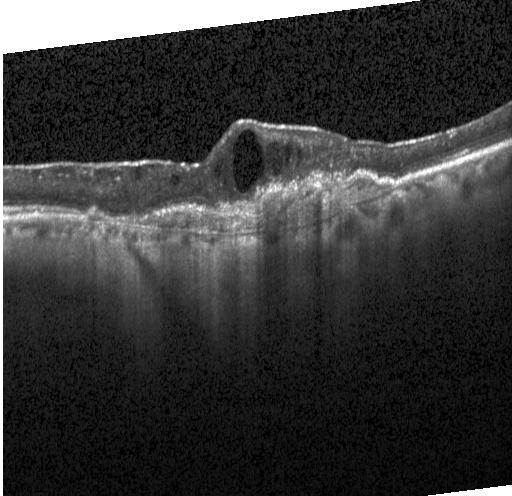

OCT B-scan — Finding: choroidal neovascularization (CNV).